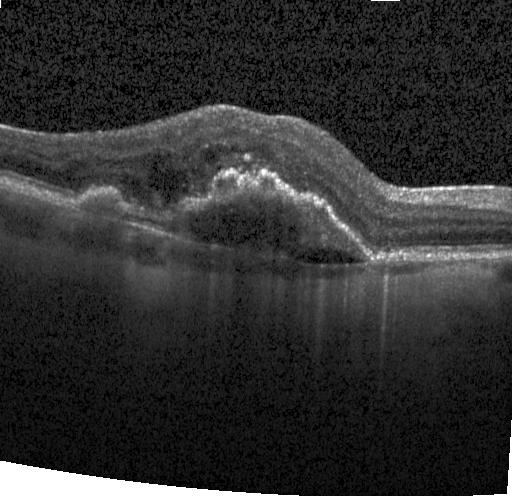 Through the macula. Retinal OCT cross-section. SD-OCT.
OCT finding: choroidal neovascularization.